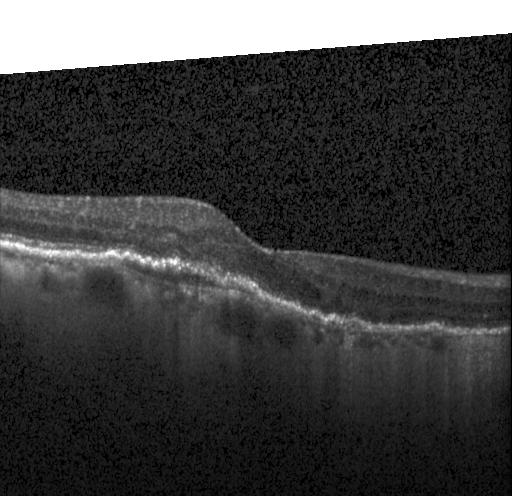 Diagnosis: CNV.